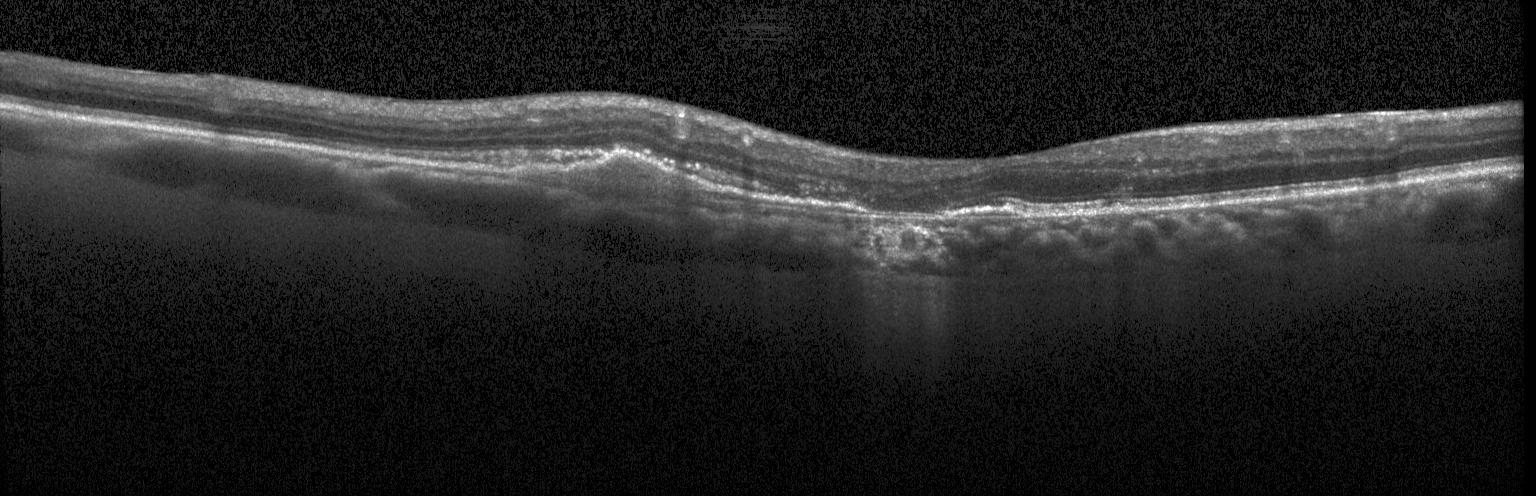

Diagnosis: CNV.